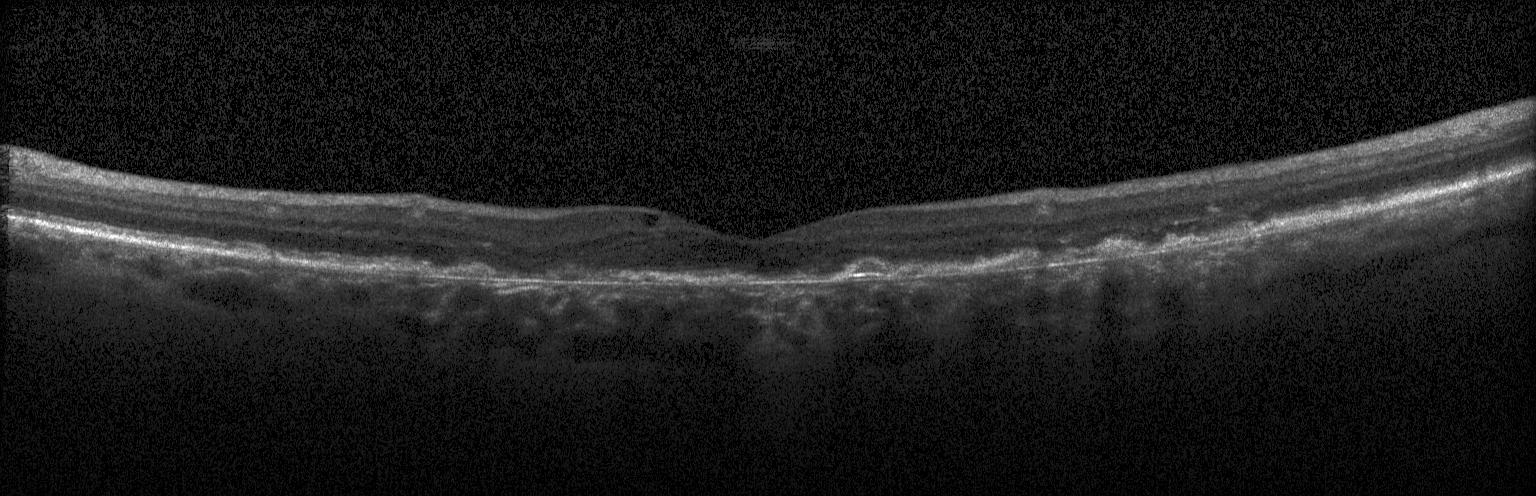 Finding: choroidal neovascularization.